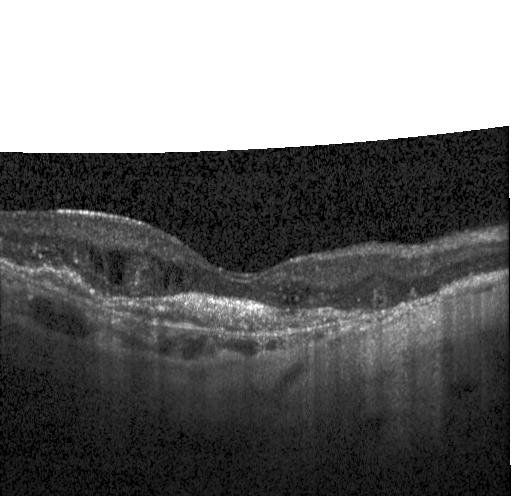 Heidelberg Spectralis. Retinal OCT cross-section. Spectral-domain OCT. Fovea-centered. Diagnosis: a choroidal neovascular membrane.